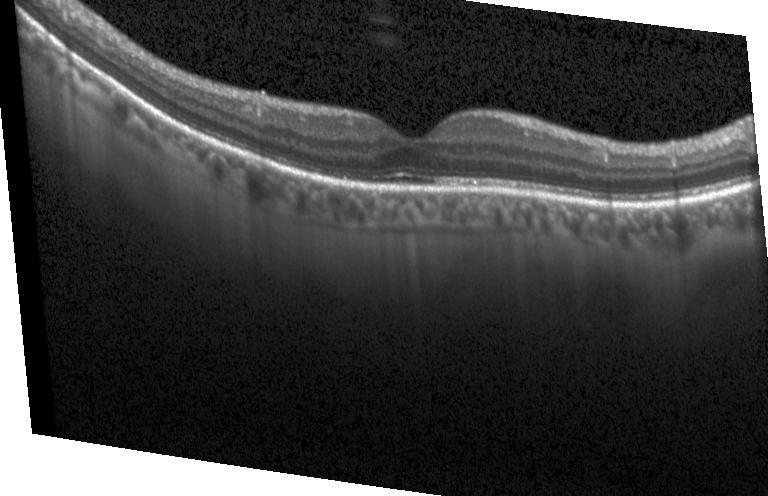 Centered on the fovea, optical coherence tomography B-scan, SD-OCT
This B-scan demonstrates neither choroidal neovascularization, diabetic macular edema, nor drusen.